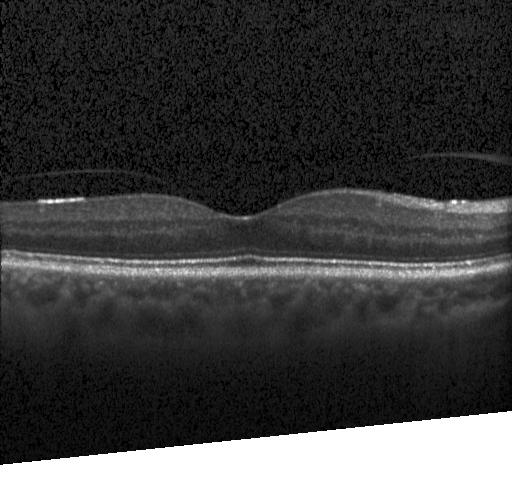 Centered on the fovea, optical coherence tomography scan
Assessment: no evidence of choroidal neovascularization, diabetic macular edema, or drusen.